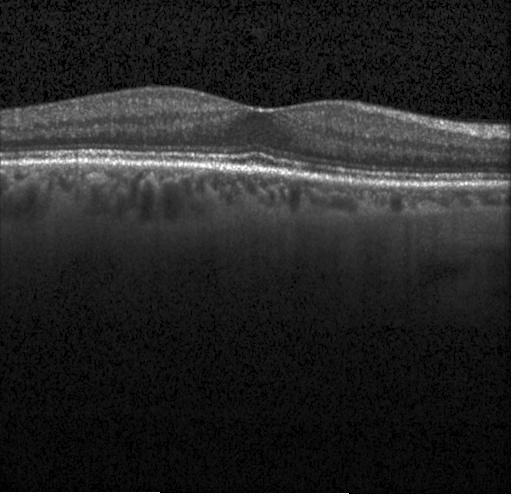 Macular scan. OCT line scan
Finding: neither choroidal neovascularization, diabetic macular edema, nor drusen.